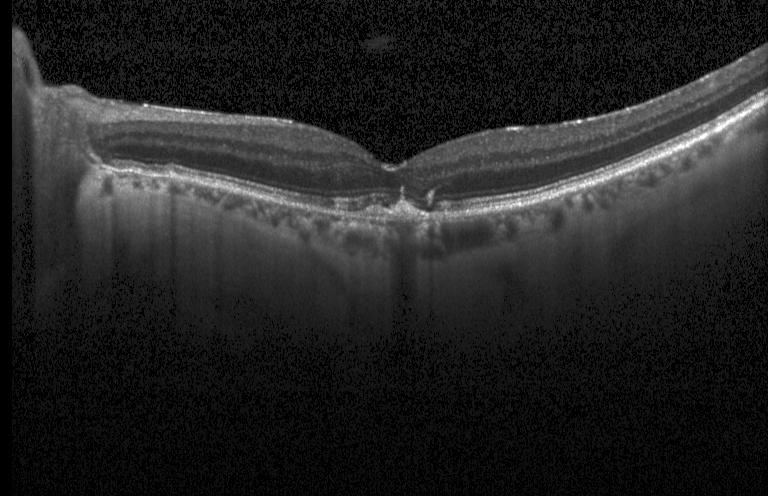 Spectral-domain optical coherence tomography. OCT B-scan. Acquired on a Heidelberg Spectralis. Fovea-centered — Finding: choroidal neovascularization (CNV).